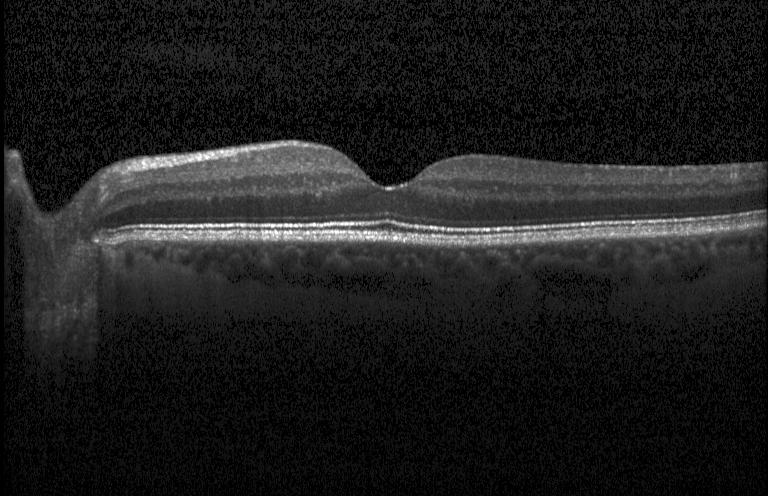 Retinal OCT B-scan · spectral-domain OCT
The scan shows no CNV, no DME, and no drusen.